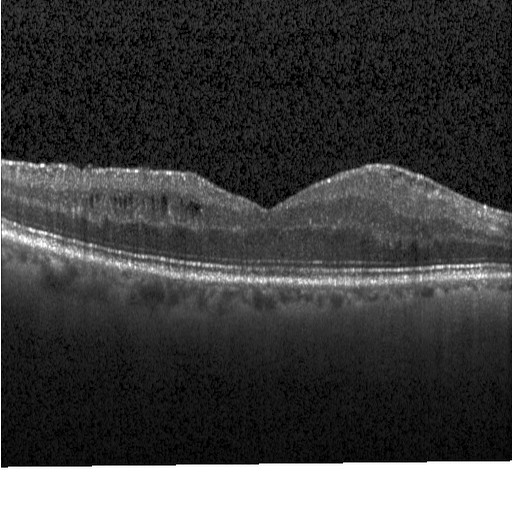 OCT B-scan showing DME.